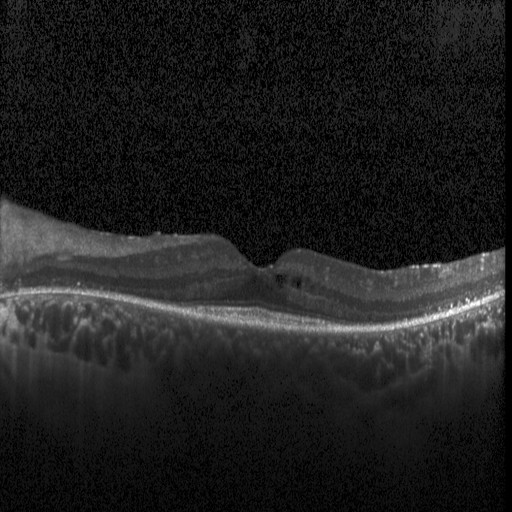 OCT finding: DME.